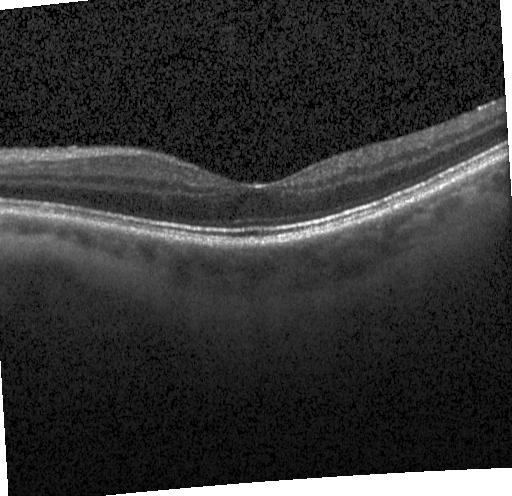
Retinal OCT cross-section. Acquired on a Heidelberg Spectralis. SD-OCT. Fovea-centered.
Impression: neither choroidal neovascularization, diabetic macular edema, nor drusen.